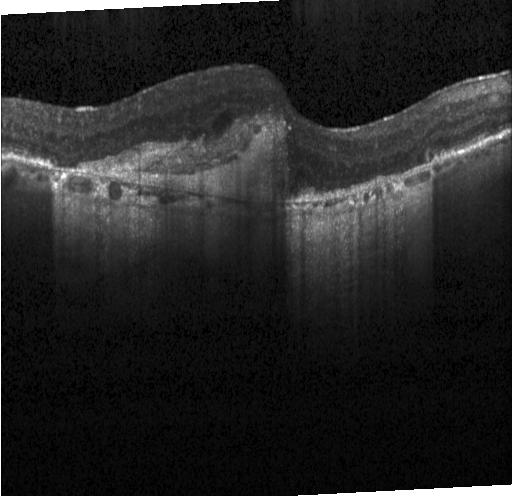 OCT B-scan — A choroidal neovascular membrane.